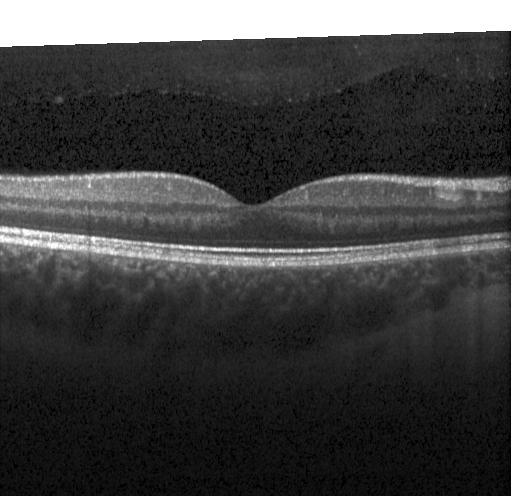

Spectral-domain optical coherence tomography, OCT B-scan. Impression: no choroidal neovascularization, diabetic macular edema, or drusen.